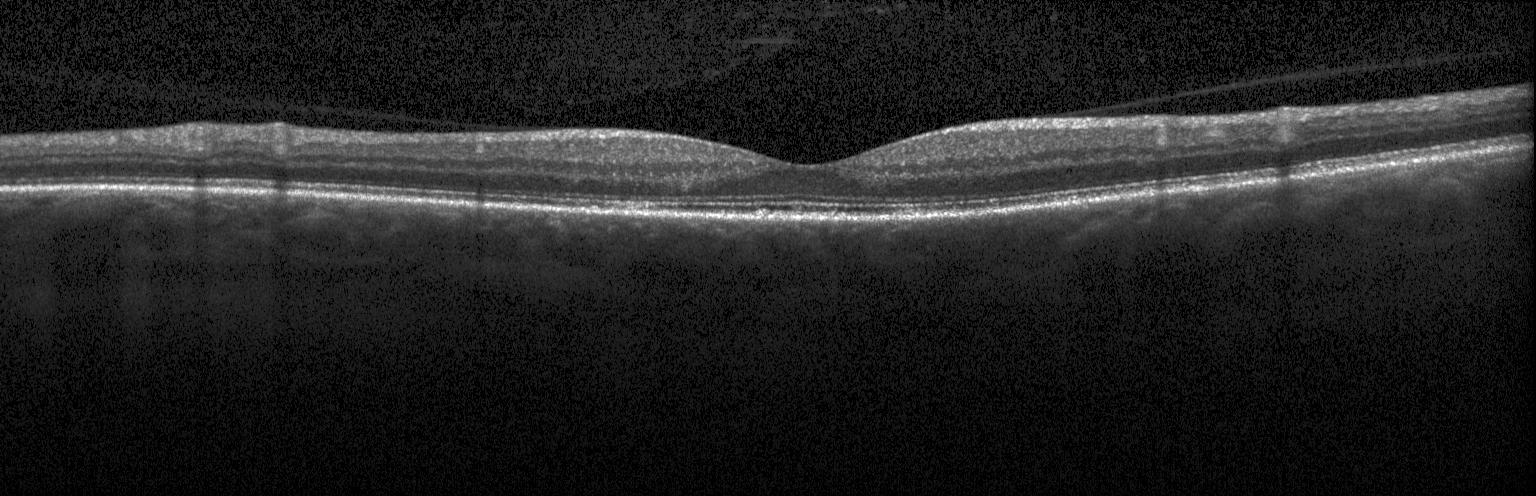
Retinal OCT cross-section.
Diagnosis: no evidence of CNV, DME, or drusen.